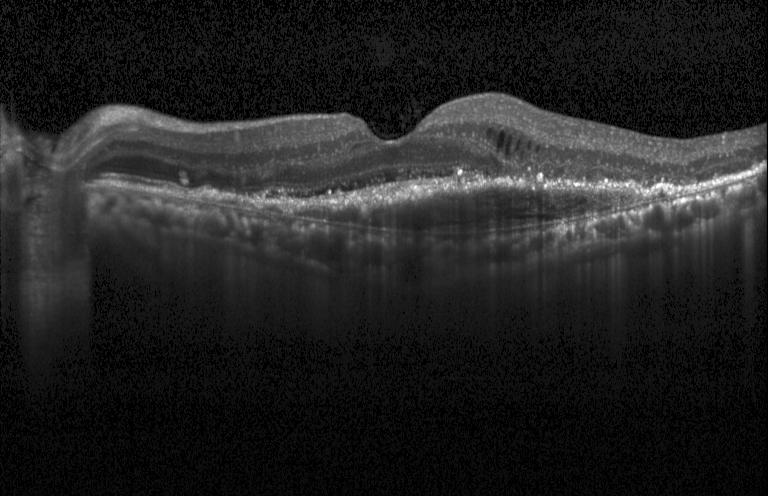

OCT line scan · instrument: Heidelberg Spectralis.
CNV.